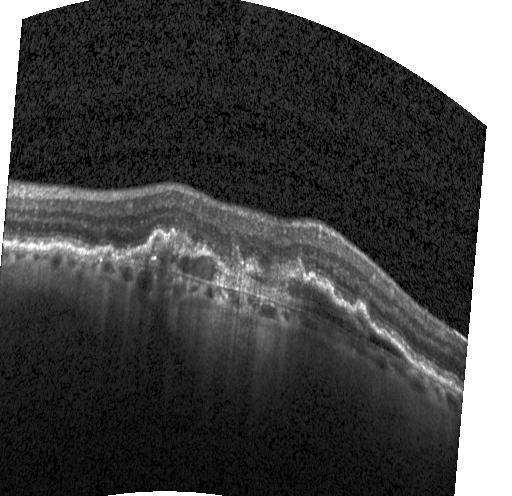

Spectral-domain OCT. Through the macula. Optical coherence tomography scan
OCT finding: a choroidal neovascular membrane.